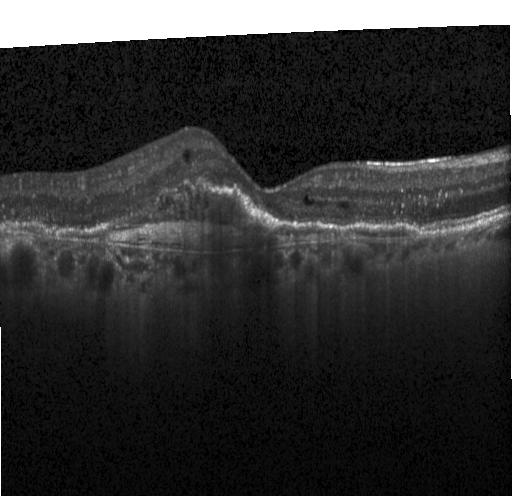

Instrument: Heidelberg Spectralis. Spectral-domain optical coherence tomography. Horizontal scan through the fovea. OCT line scan. OCT finding: CNV.